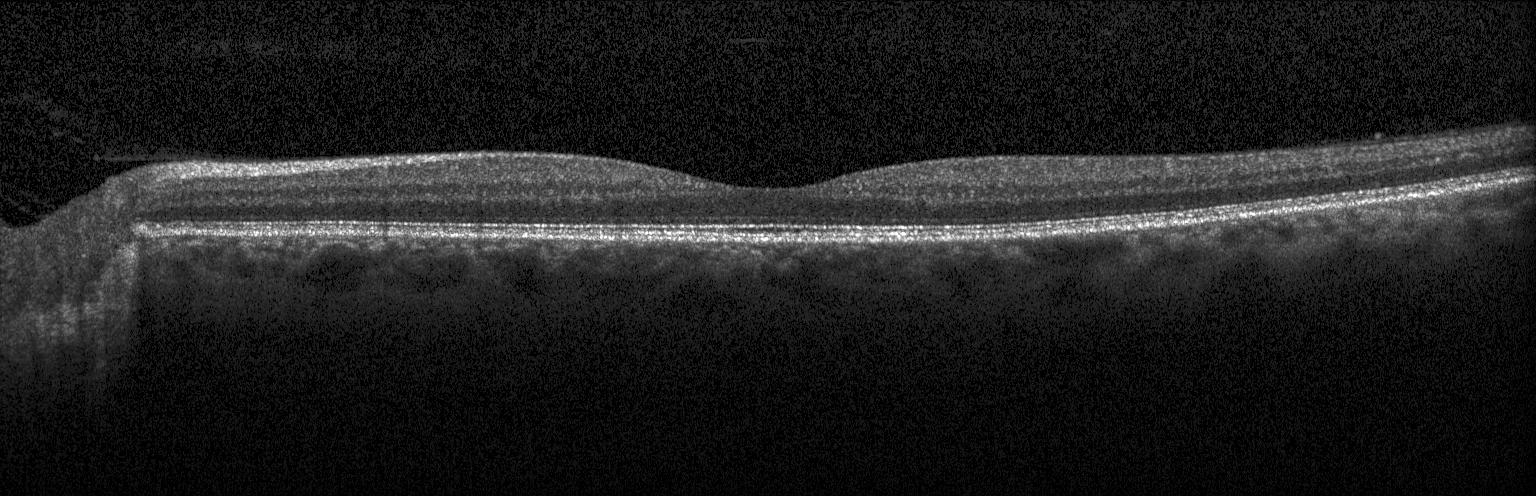
Optical coherence tomography scan.
This B-scan demonstrates no CNV, DME, or drusen.